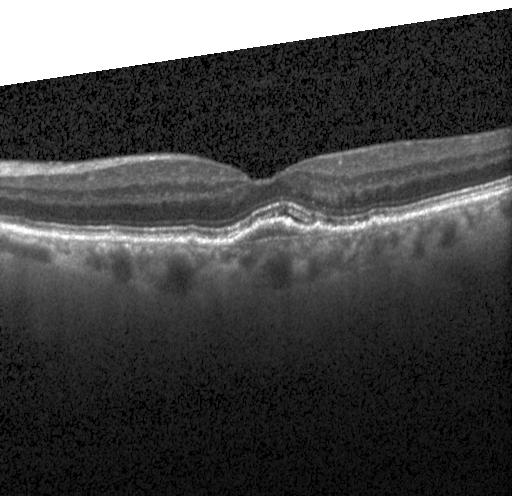

Impression: choroidal neovascularization (CNV).